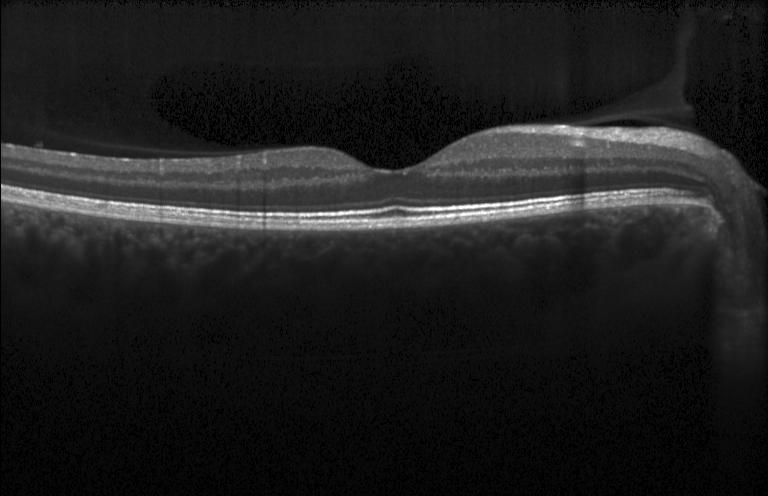

Spectral-domain OCT, Heidelberg Spectralis, OCT line scan, through the macula — Finding: no choroidal neovascularization, no diabetic macular edema, and no drusen.